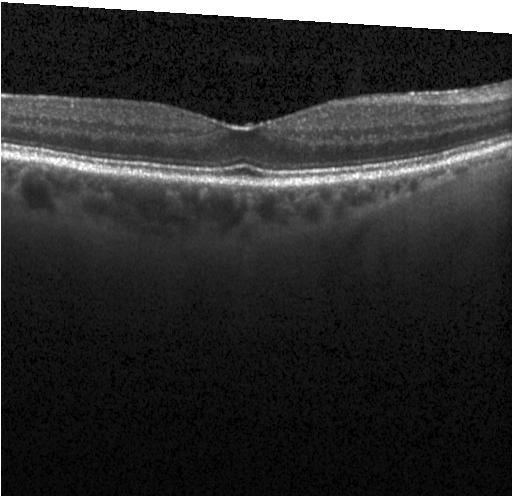 OCT scan showing no CNV, DME, or drusen.